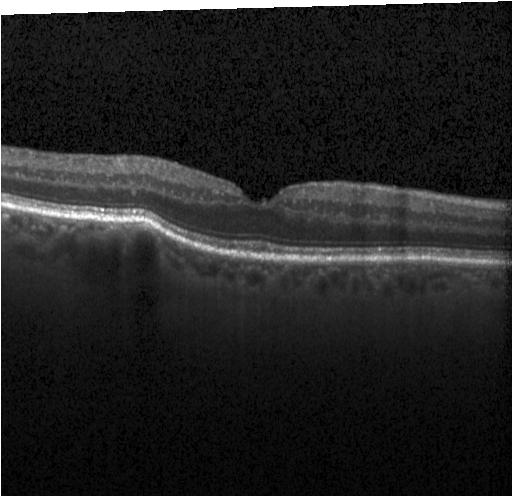
OCT B-scan; Heidelberg Spectralis OCT system; fovea-centered — Diagnosis: no evidence of choroidal neovascularization, diabetic macular edema, or drusen.